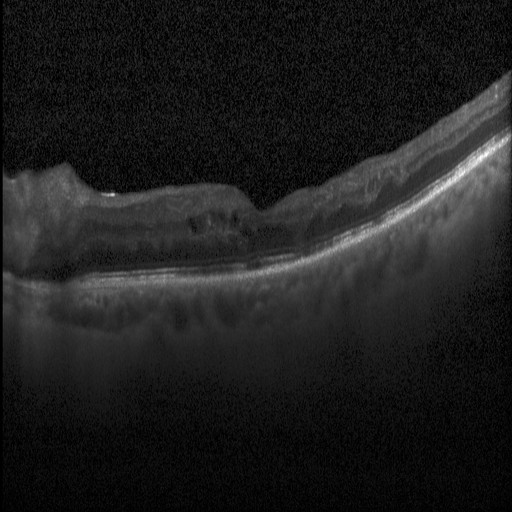 Macular OCT: DME.